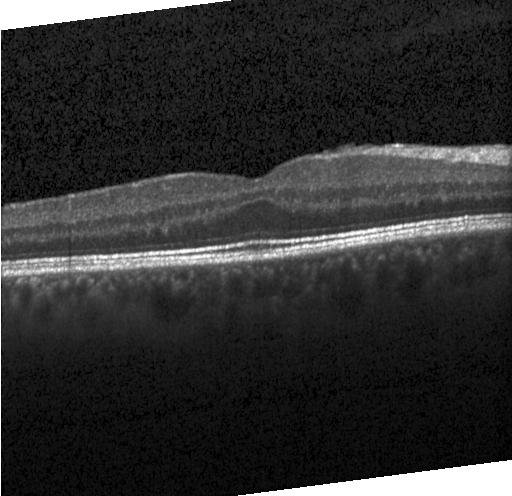 Heidelberg Spectralis. Spectral-domain optical coherence tomography. Horizontal scan through the fovea. OCT B-scan
Assessment: no evidence of choroidal neovascularization, diabetic macular edema, or drusen.